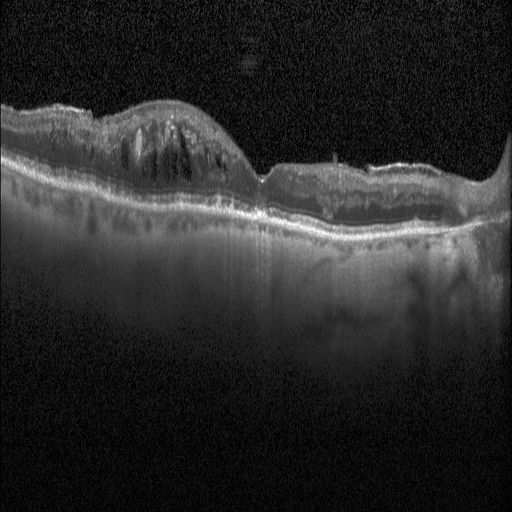

OCT B-scan — This B-scan demonstrates diabetic macular edema.